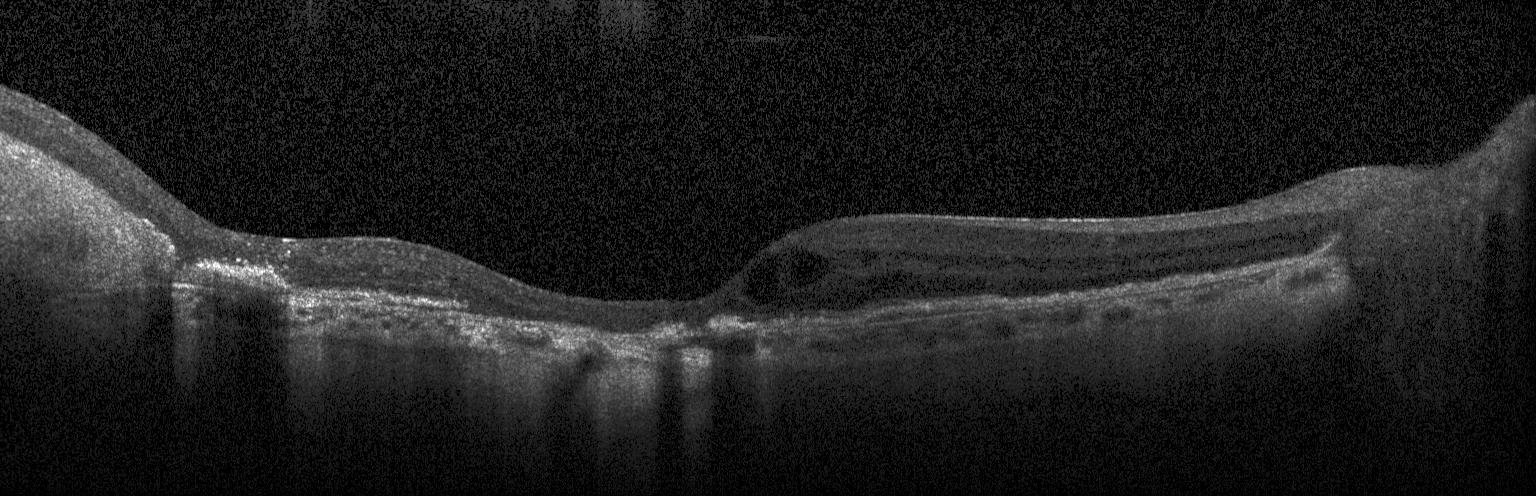

OCT line scan · SD-OCT · Heidelberg Spectralis OCT system · macular scan. Diagnosis: a choroidal neovascular membrane.